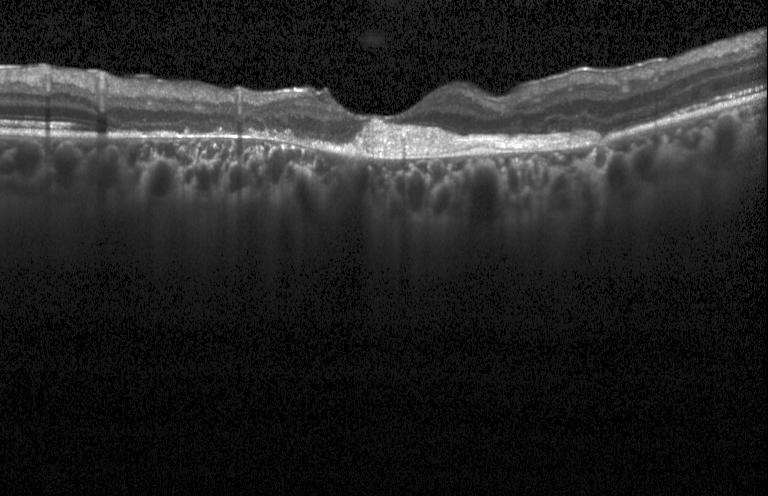 Instrument: Heidelberg Spectralis; SD-OCT; OCT line scan — Macular OCT: choroidal neovascularization.